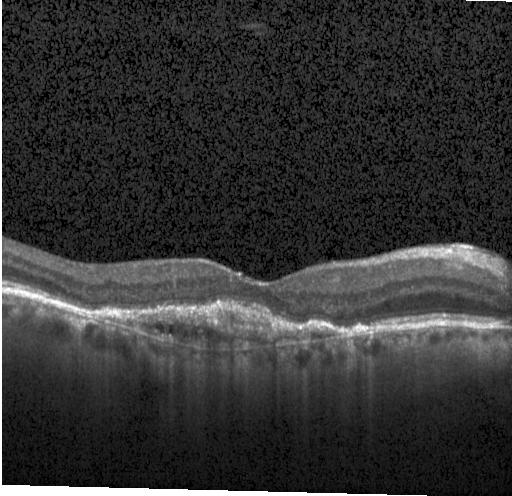 Spectral-domain OCT. Optical coherence tomography scan. Acquired on a Heidelberg Spectralis — Finding: a choroidal neovascular membrane.